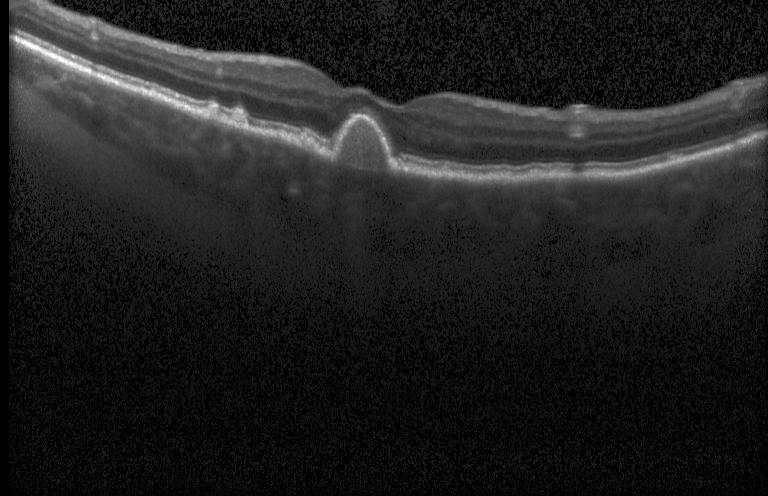

OCT line scan — The scan shows sub-RPE drusenoid deposits.